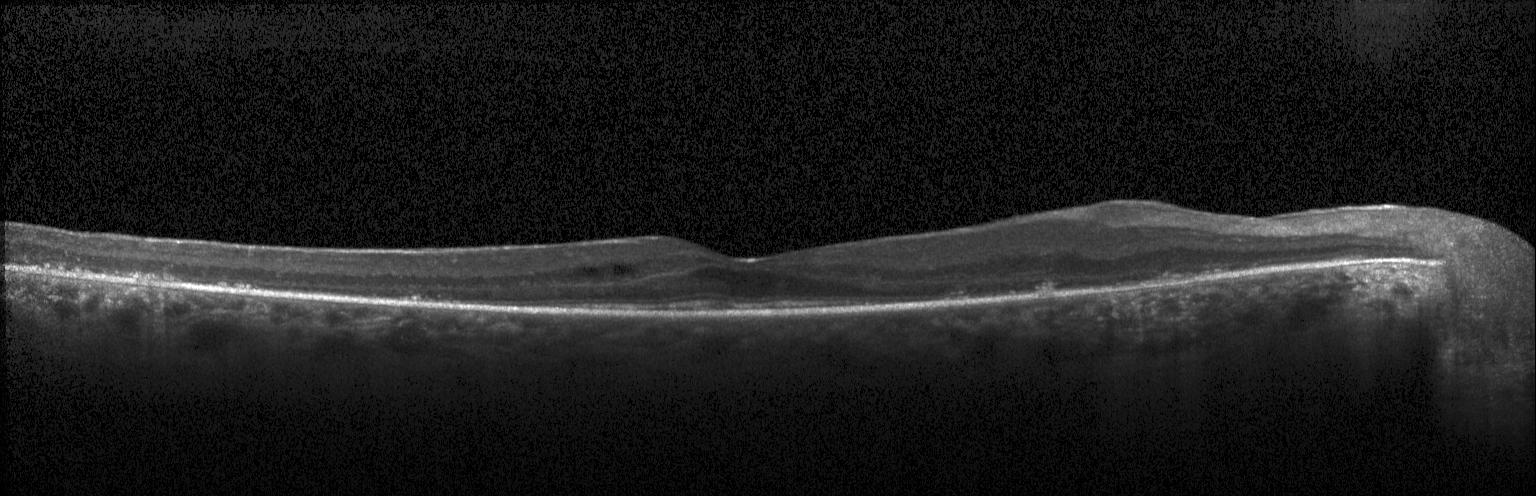

The scan shows diabetic macular edema (DME).